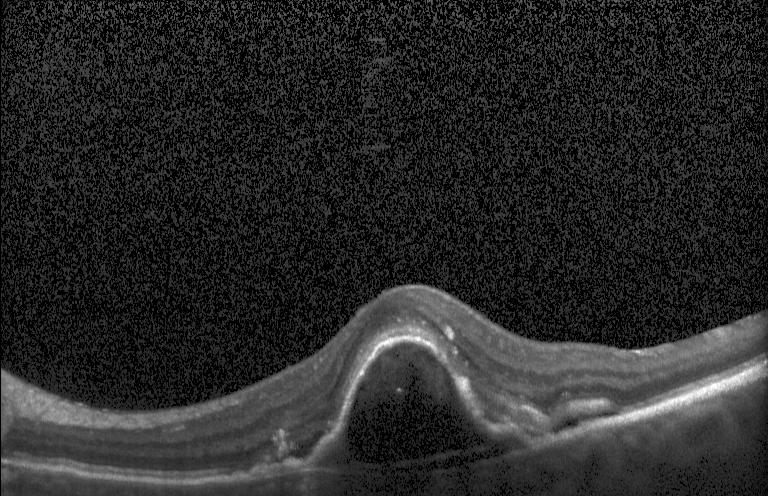 OCT line scan.
The scan shows a choroidal neovascular membrane.